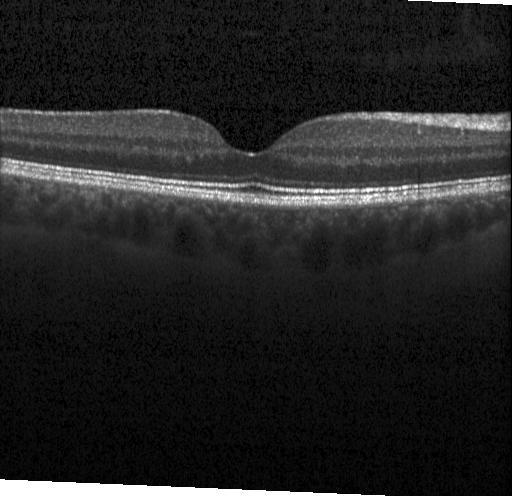

OCT line scan. Macular OCT: neither CNV, DME, nor drusen.